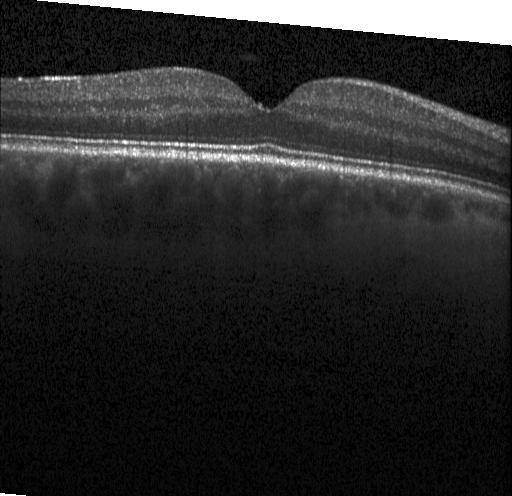
Assessment: no evidence of CNV, DME, or drusen.